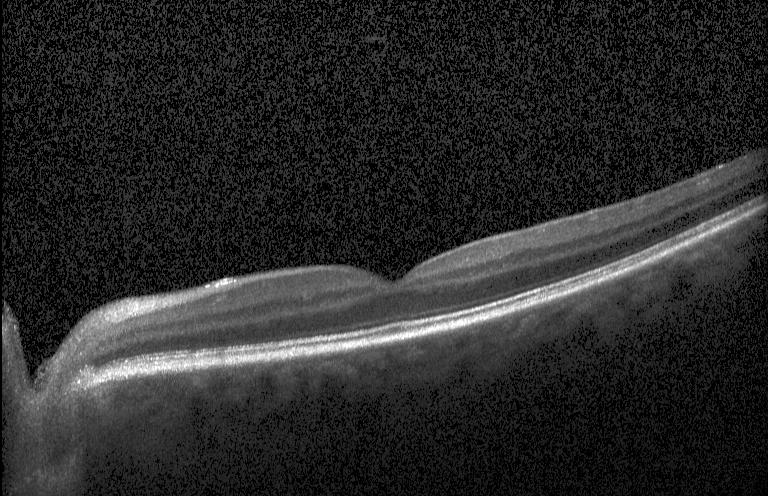

OCT scan showing no evidence of choroidal neovascularization, diabetic macular edema, or drusen.